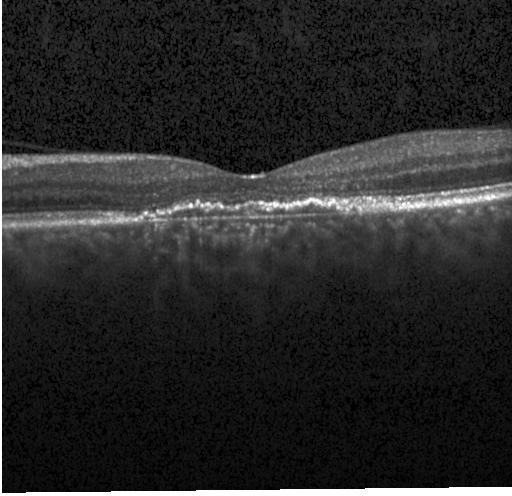
Through the macula; retinal OCT B-scan; Heidelberg Spectralis; SD-OCT.
Assessment: a choroidal neovascular membrane.